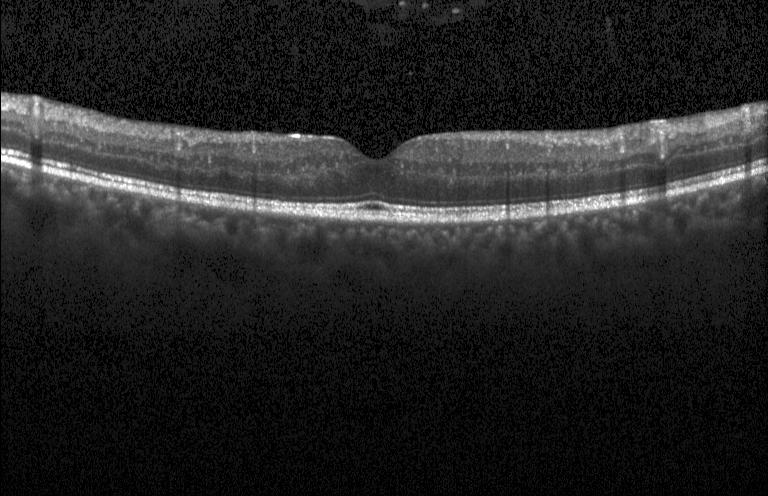 OCT finding: no choroidal neovascularization, diabetic macular edema, or drusen.